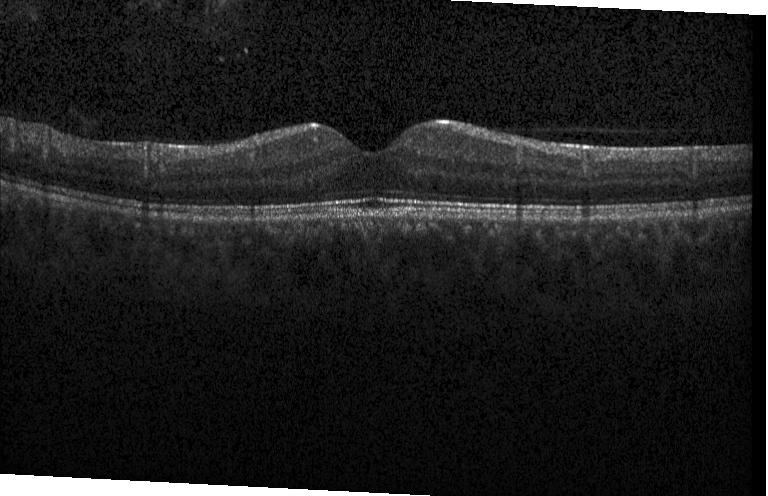
Diagnosis: no evidence of choroidal neovascularization, diabetic macular edema, or drusen.